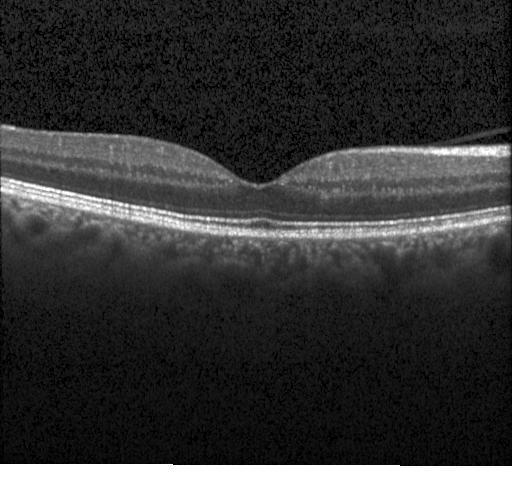

Optical coherence tomography scan; acquired on a Heidelberg Spectralis.
Finding: no choroidal neovascularization, diabetic macular edema, or drusen.